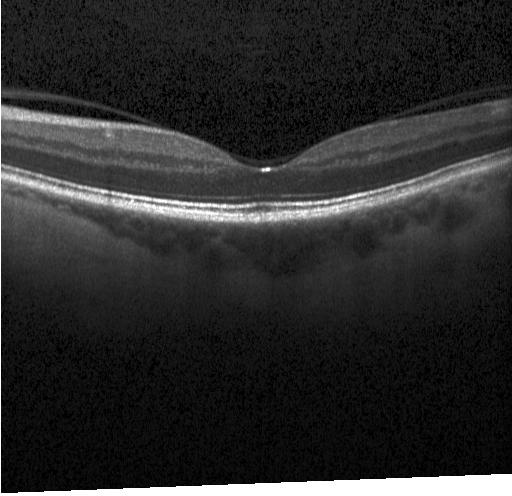
Centered on the fovea. Optical coherence tomography B-scan. Spectral-domain optical coherence tomography. Instrument: Heidelberg Spectralis.
The scan shows no choroidal neovascularization, no diabetic macular edema, and no drusen.